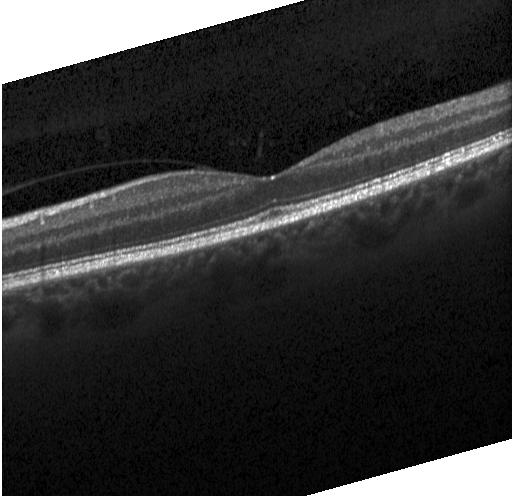 OCT B-scan showing no CNV, DME, or drusen.